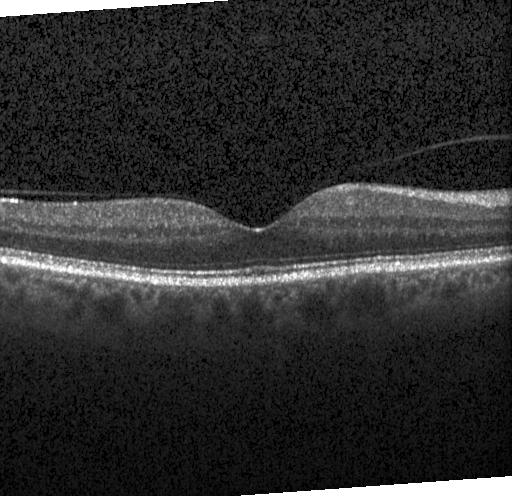 OCT line scan, spectral-domain OCT, centered on the fovea. Macular OCT: no CNV, no DME, and no drusen.